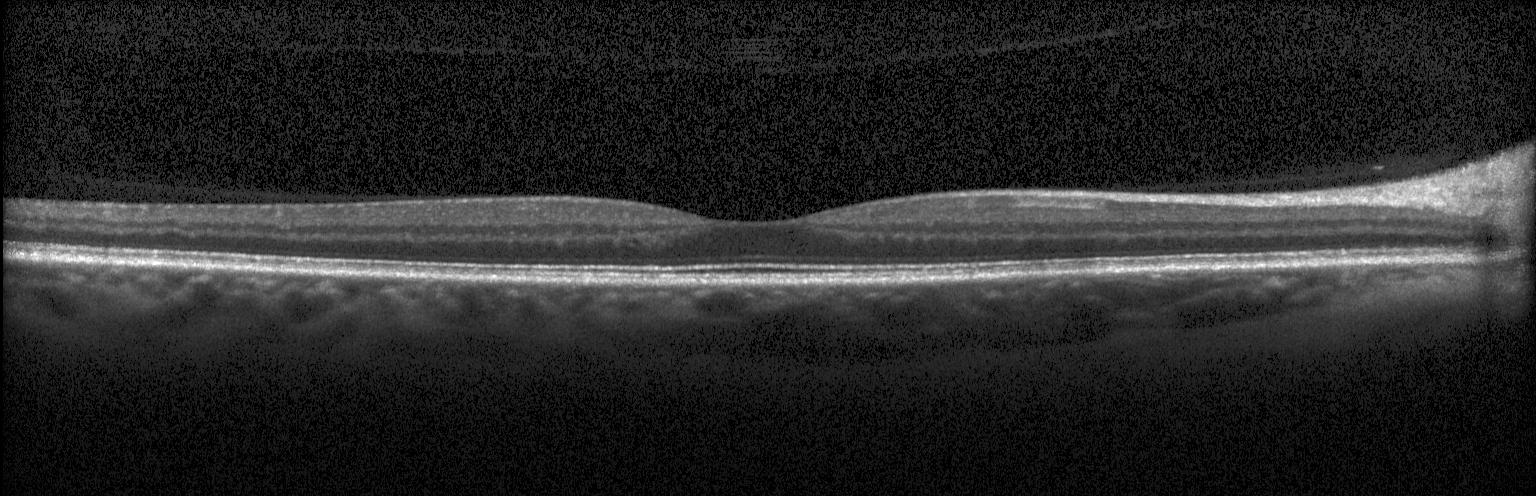
Retinal OCT B-scan. Diagnosis: no choroidal neovascularization, no diabetic macular edema, and no drusen.